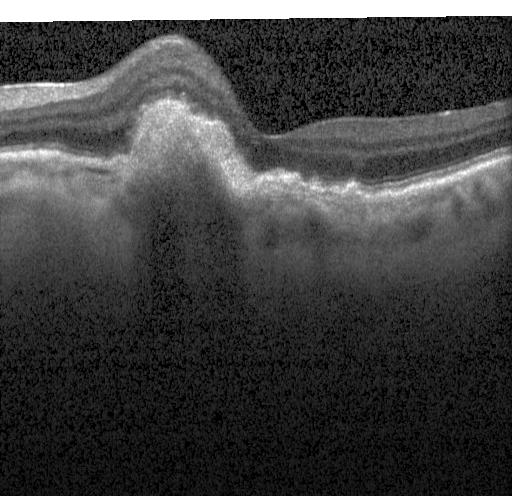

OCT B-scan showing CNV.